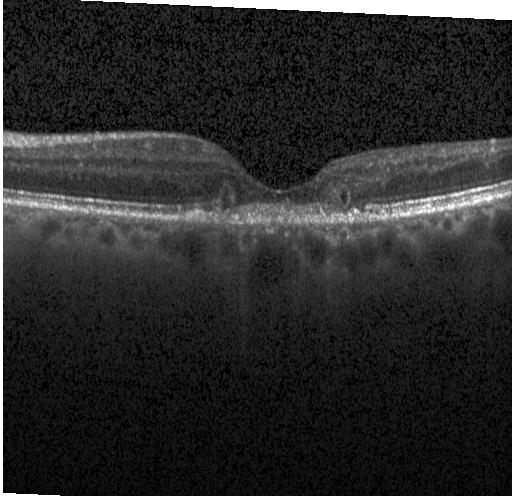

OCT finding: choroidal neovascularization (CNV).